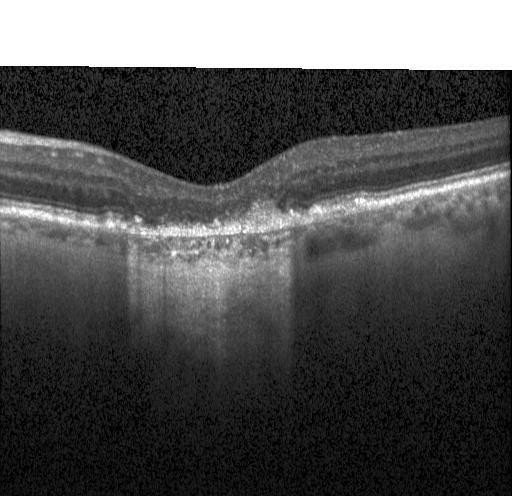 Horizontal scan through the fovea. Instrument: Heidelberg Spectralis. OCT line scan. SD-OCT. Diagnosis: choroidal neovascularization.